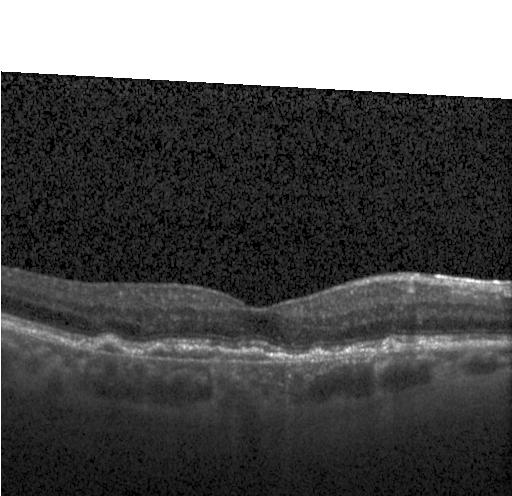 Optical coherence tomography B-scan
Macular OCT: choroidal neovascularization.